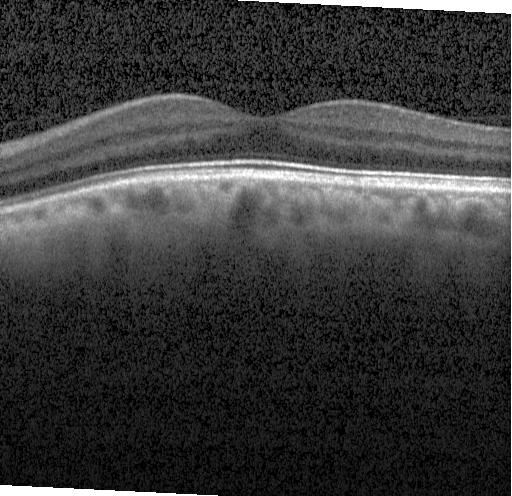
Finding: no CNV, DME, or drusen.